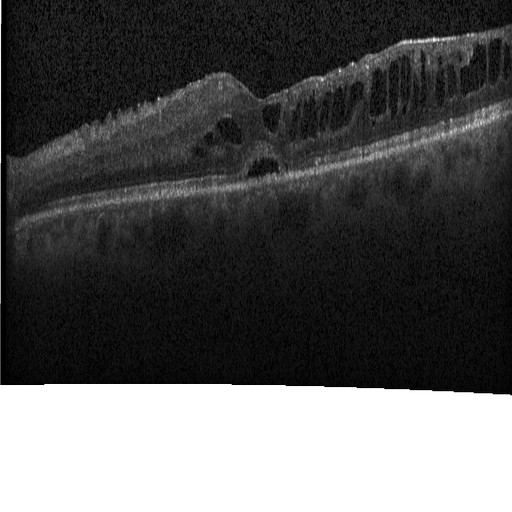
Spectral-domain OCT. Heidelberg Spectralis. OCT line scan. Through the macula — Dx: DME.